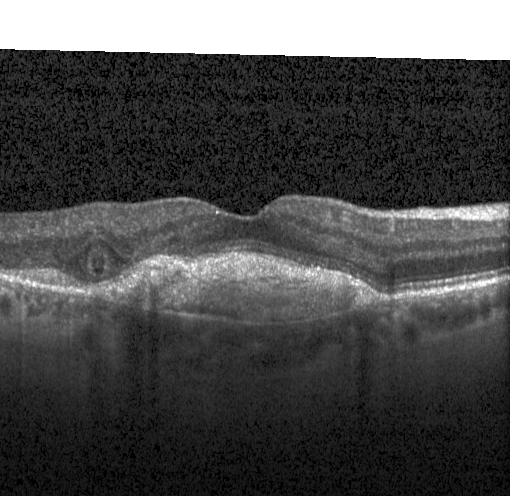
Diagnosis: a choroidal neovascular membrane.